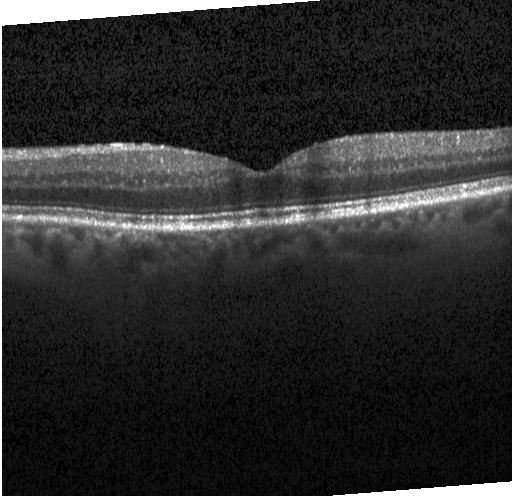 Horizontal scan through the fovea. Heidelberg Spectralis. Retinal OCT B-scan
Dx: no choroidal neovascularization, diabetic macular edema, or drusen.